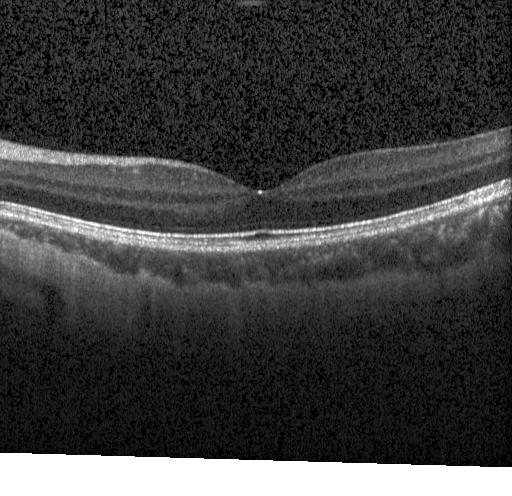
SD-OCT; centered on the fovea; OCT line scan — Finding: no evidence of CNV, DME, or drusen.